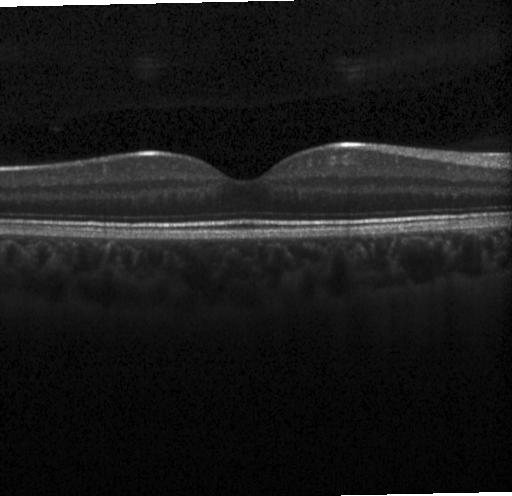
Centered on the fovea, Heidelberg Spectralis, OCT line scan. Impression: no evidence of choroidal neovascularization, diabetic macular edema, or drusen.